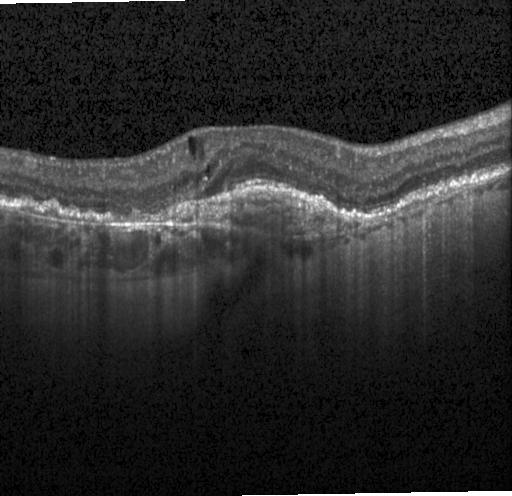 OCT finding: a choroidal neovascular membrane.